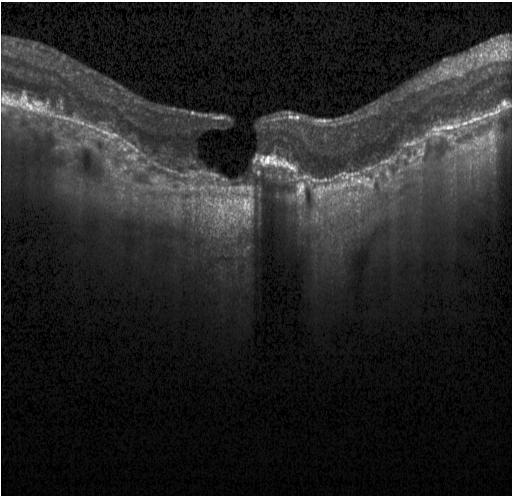 Acquired on a Heidelberg Spectralis, retinal OCT B-scan — Macular OCT: choroidal neovascularization (CNV).